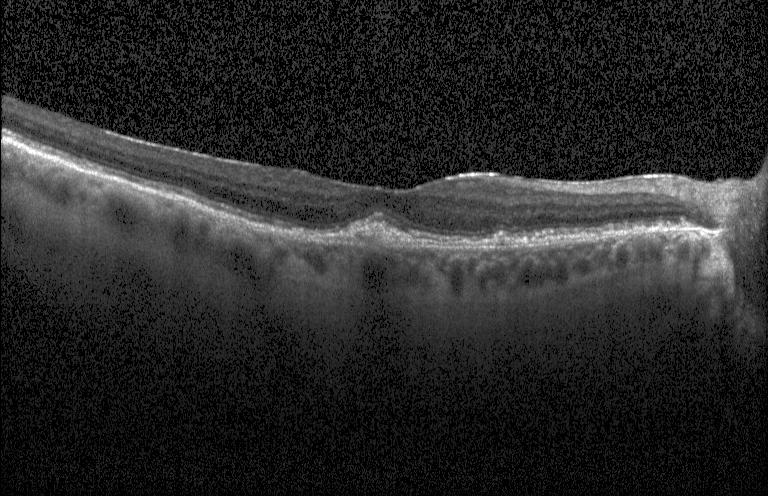

Retinal OCT cross-section; spectral-domain OCT.
Assessment: a choroidal neovascular membrane.